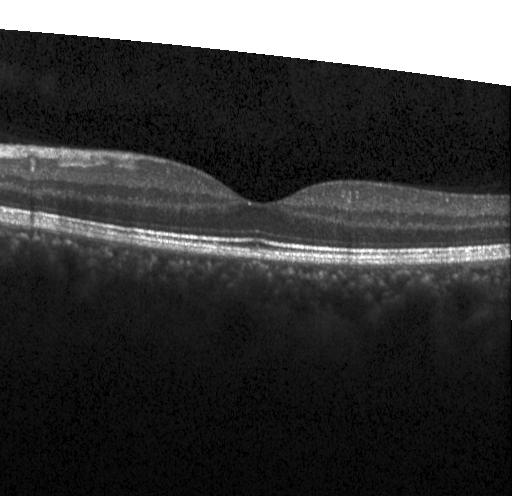 Spectral-domain optical coherence tomography. OCT line scan. Centered on the fovea. Heidelberg Spectralis OCT system
Impression: no evidence of choroidal neovascularization, diabetic macular edema, or drusen.